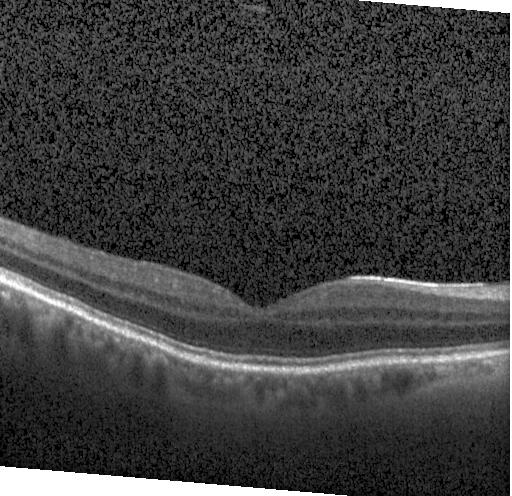 Macular OCT: no evidence of choroidal neovascularization, diabetic macular edema, or drusen.